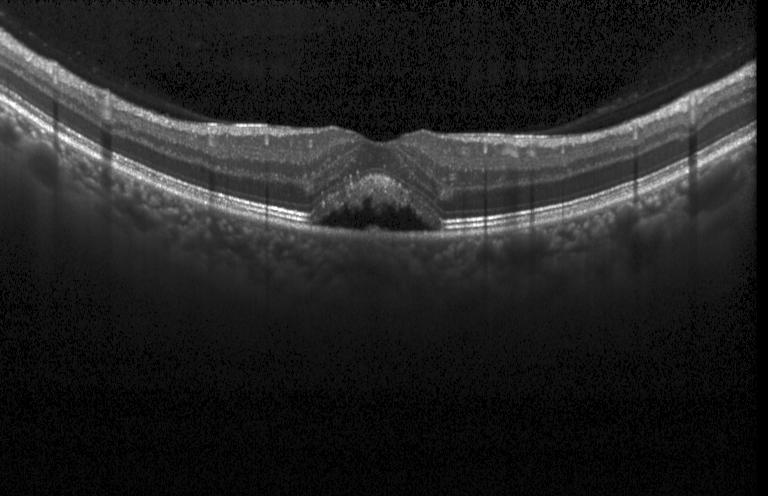 SD-OCT; retinal OCT B-scan; fovea-centered. Diagnosis: a choroidal neovascular membrane.